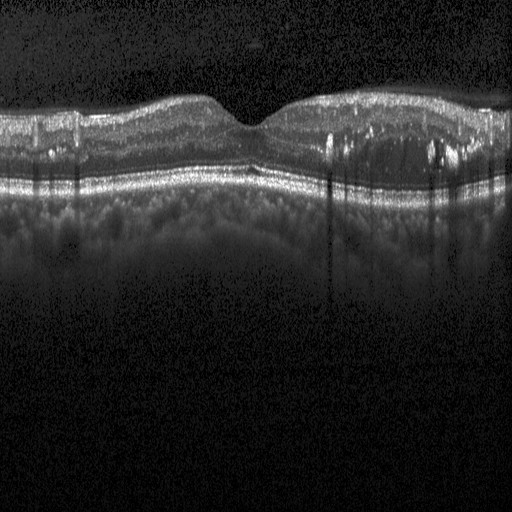
Retinal OCT B-scan.
Impression: diabetic macular edema (DME).